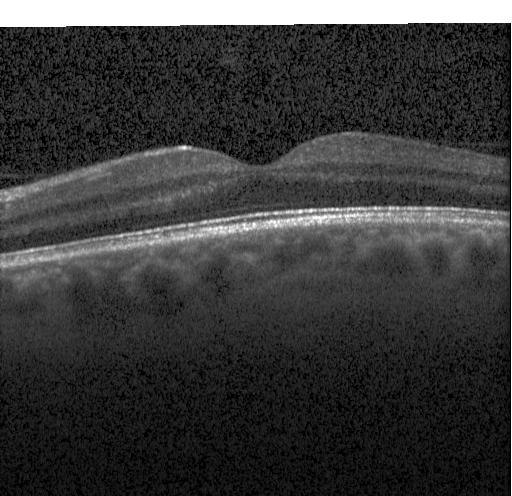
Macular OCT demonstrating neither choroidal neovascularization, diabetic macular edema, nor drusen.